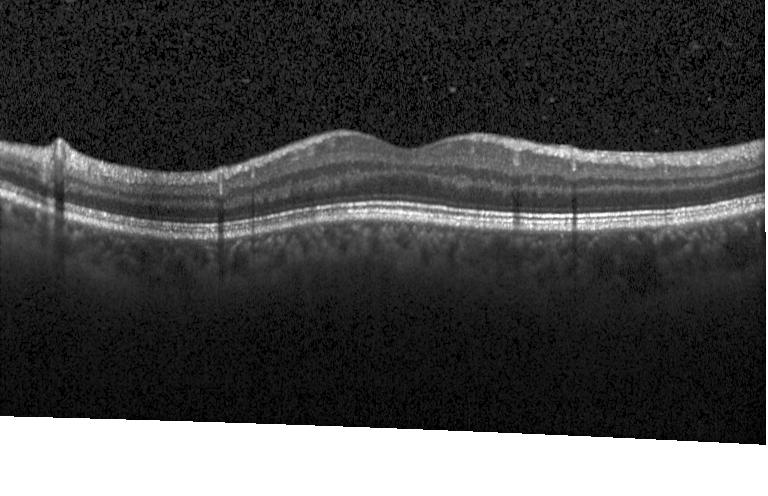
Retinal OCT B-scan · Heidelberg Spectralis · through the macula · spectral-domain OCT.
Diagnosis: no choroidal neovascularization, no diabetic macular edema, and no drusen.